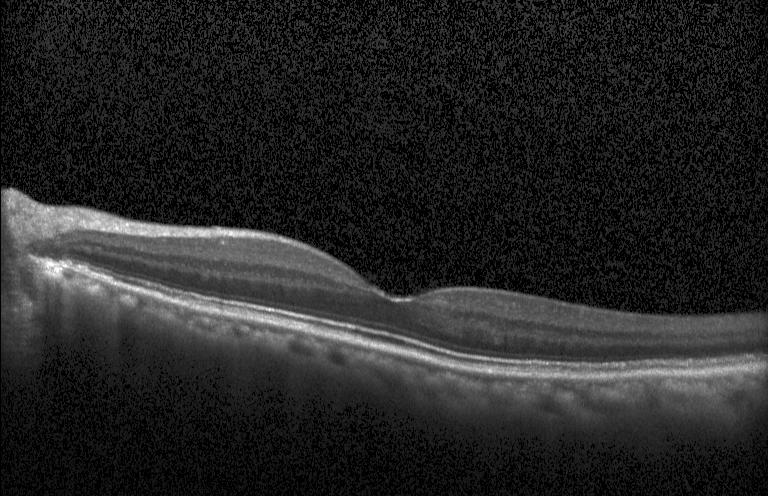 Spectral-domain optical coherence tomography · through the macula · retinal OCT B-scan. This B-scan demonstrates no CNV, no DME, and no drusen.